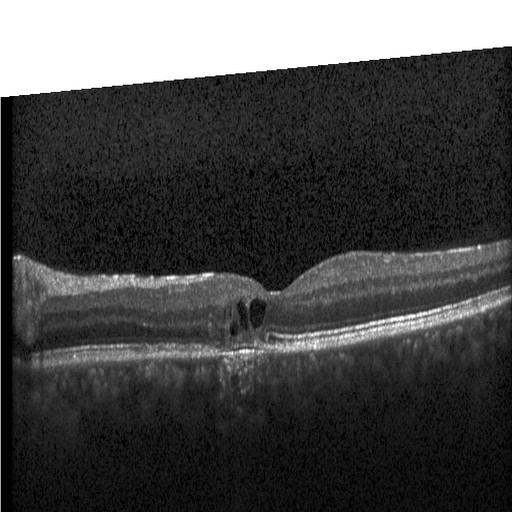
Dx: DME.